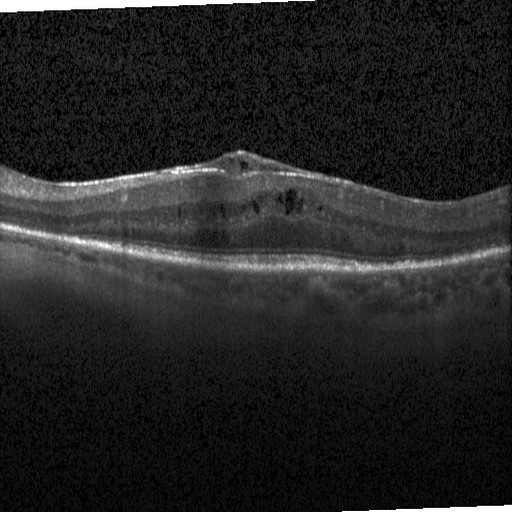

Heidelberg Spectralis OCT system · retinal OCT cross-section. Dx: diabetic macular edema.